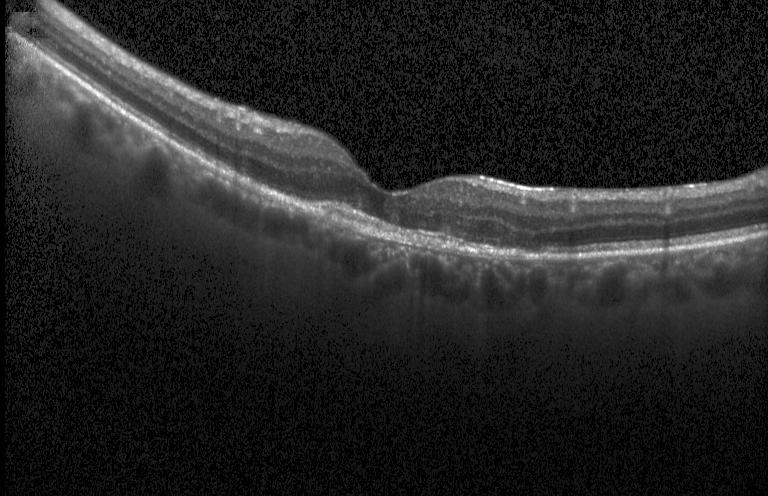 Impression: choroidal neovascularization.